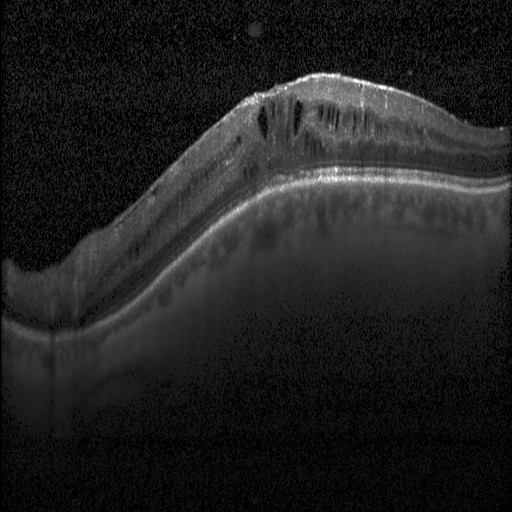

OCT scan showing diabetic macular edema (DME).